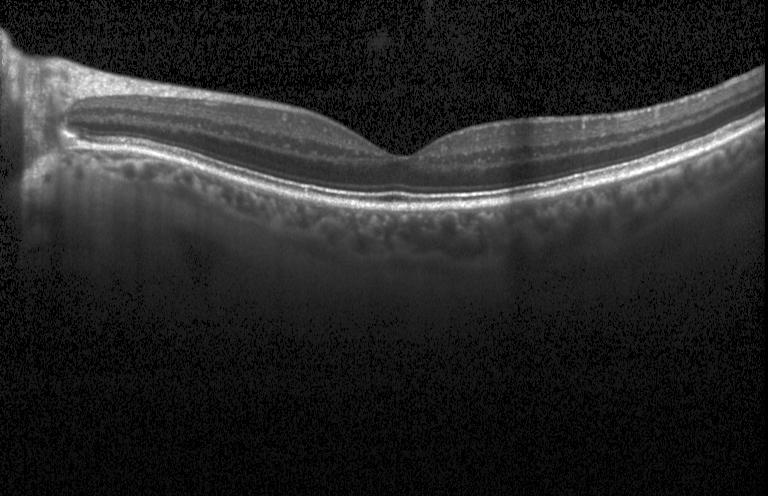
Finding: no CNV, no DME, and no drusen.